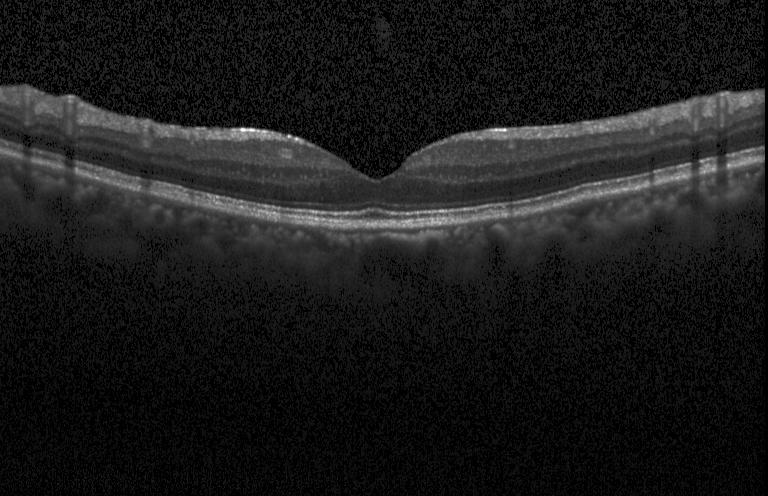 OCT B-scan showing neither choroidal neovascularization, diabetic macular edema, nor drusen.